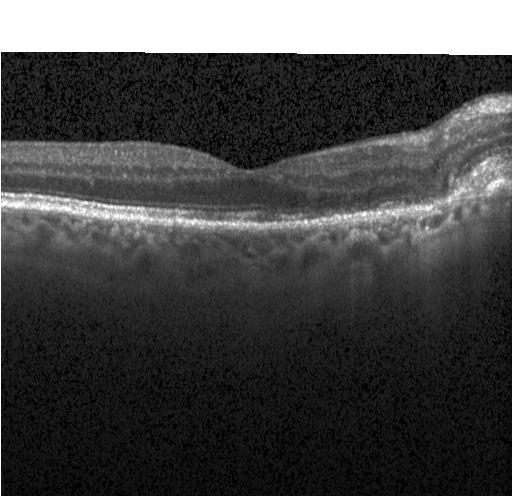 Dx: a choroidal neovascular membrane.